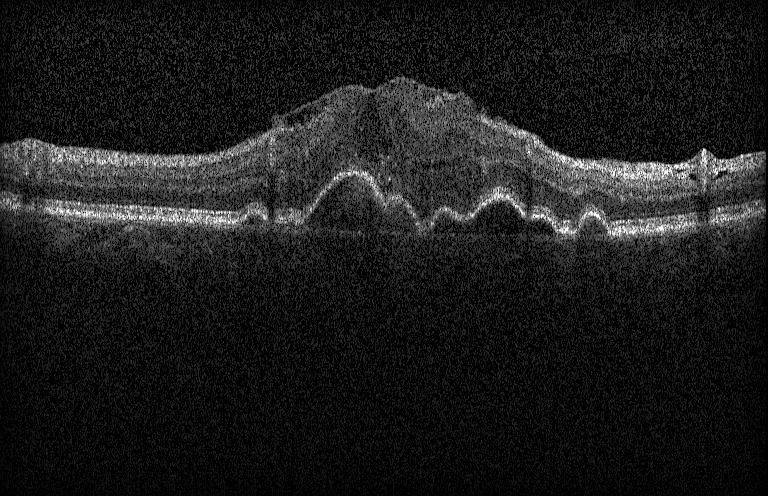
Heidelberg Spectralis. OCT B-scan
The scan shows a choroidal neovascular membrane.